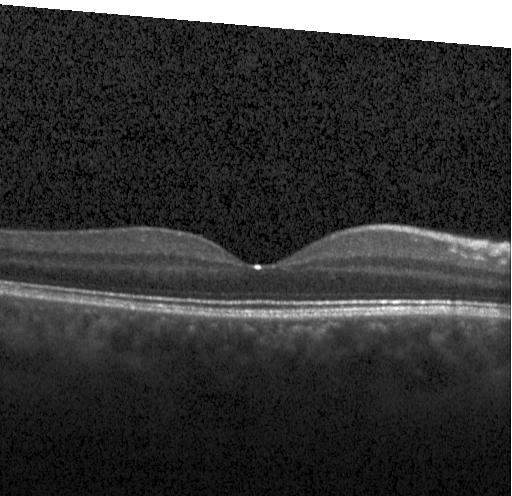
Retinal OCT B-scan · Heidelberg Spectralis OCT system · spectral-domain optical coherence tomography · fovea-centered
The scan shows no choroidal neovascularization, diabetic macular edema, or drusen.